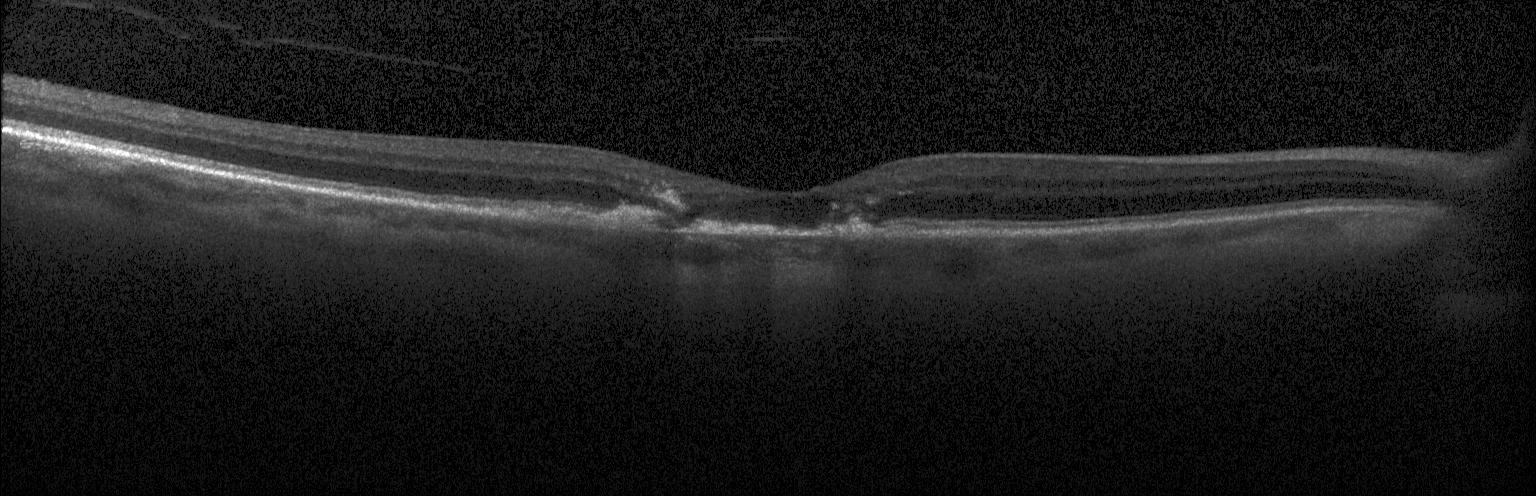 Retinal OCT cross-section; fovea-centered; Heidelberg Spectralis OCT system
A choroidal neovascular membrane.